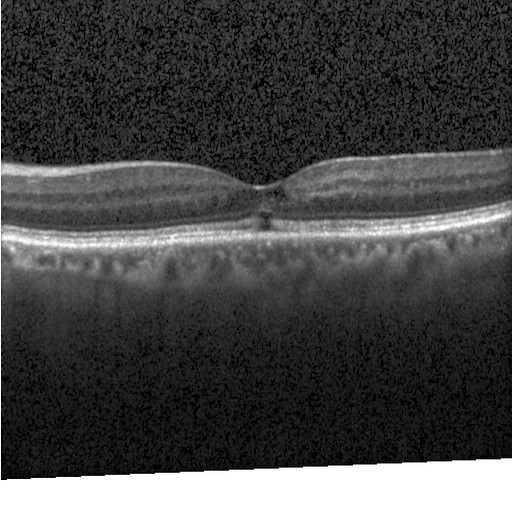
Fovea-centered · OCT B-scan
Finding: diabetic macular edema.